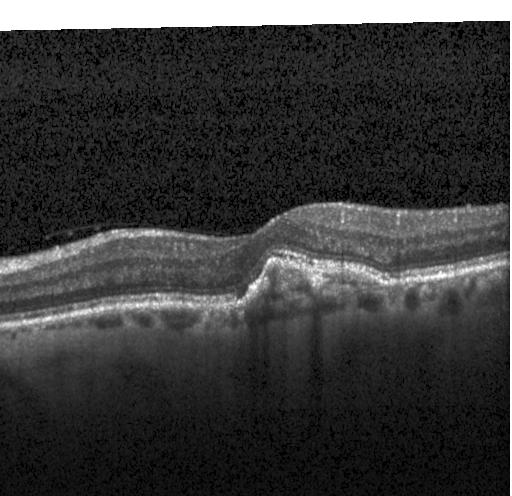
Impression: a choroidal neovascular membrane.